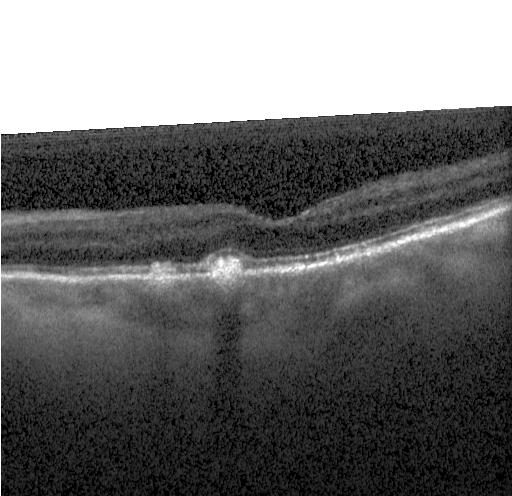

Finding: sub-RPE drusenoid deposits.